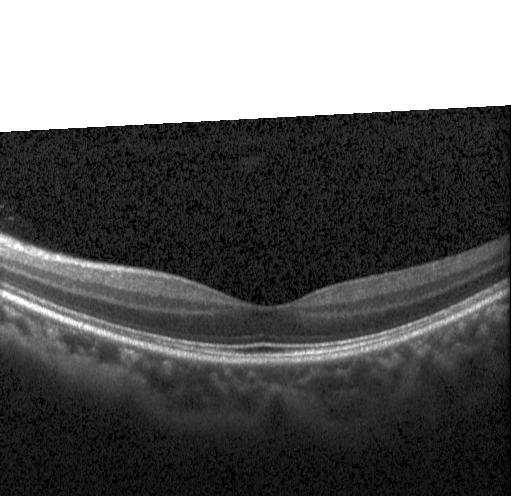 Impression: no evidence of CNV, DME, or drusen.